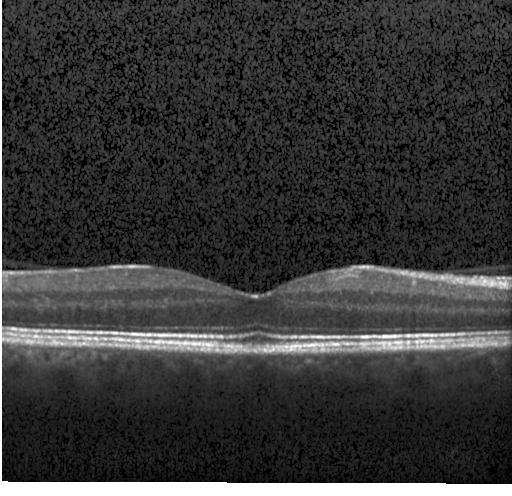

Through the macula; optical coherence tomography scan; spectral-domain optical coherence tomography; instrument: Heidelberg Spectralis.
Macular OCT: neither choroidal neovascularization, diabetic macular edema, nor drusen.